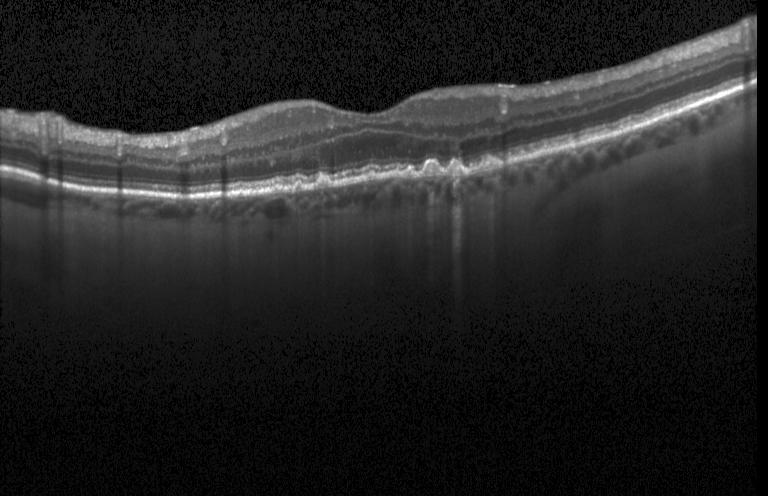
Macular OCT: sub-RPE drusenoid deposits.